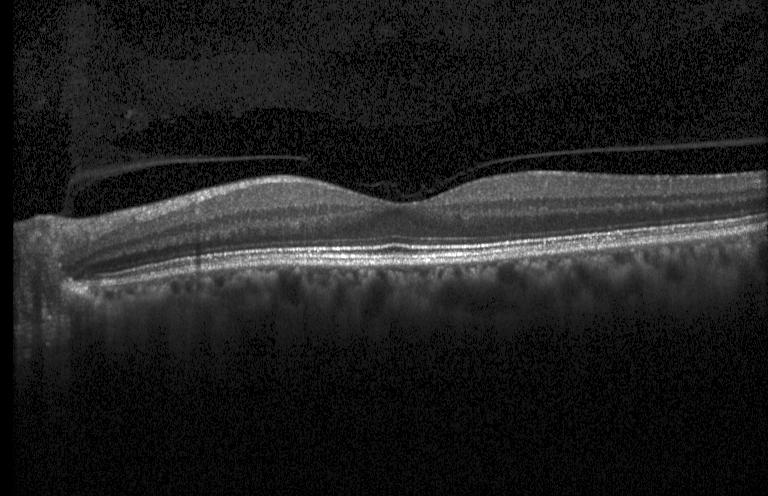 Retinal OCT B-scan — The scan shows no evidence of choroidal neovascularization, diabetic macular edema, or drusen.